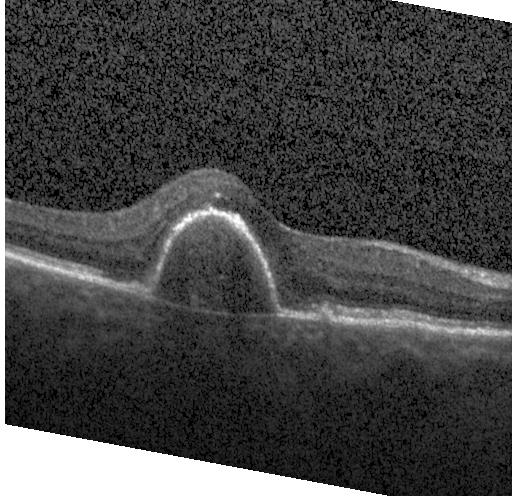

Finding: a choroidal neovascular membrane.